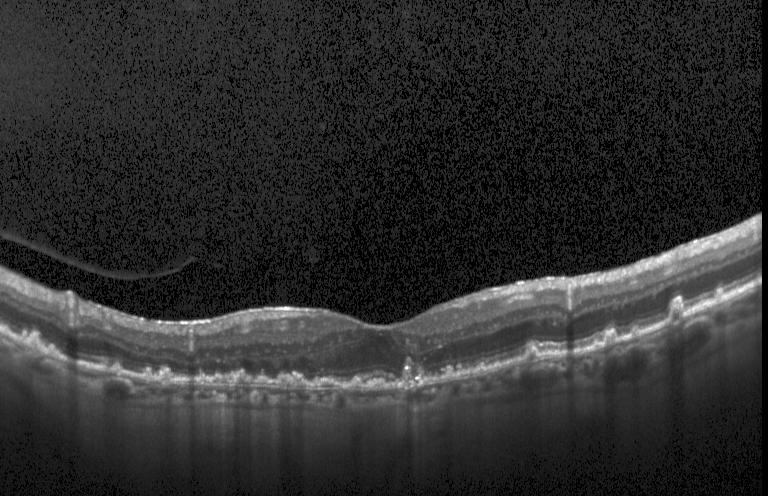 Optical coherence tomography B-scan — Impression: a choroidal neovascular membrane.